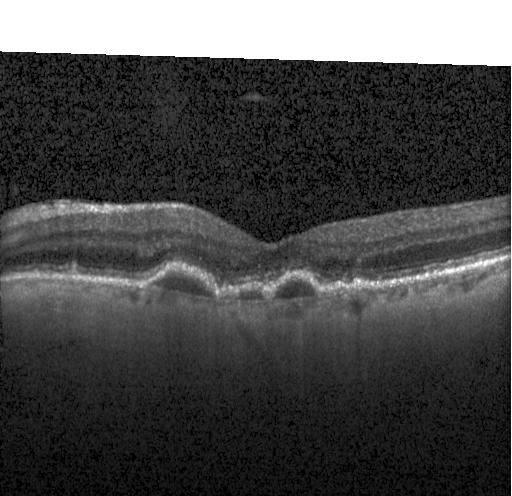
Macular scan. Retinal OCT B-scan. Dx: a choroidal neovascular membrane.